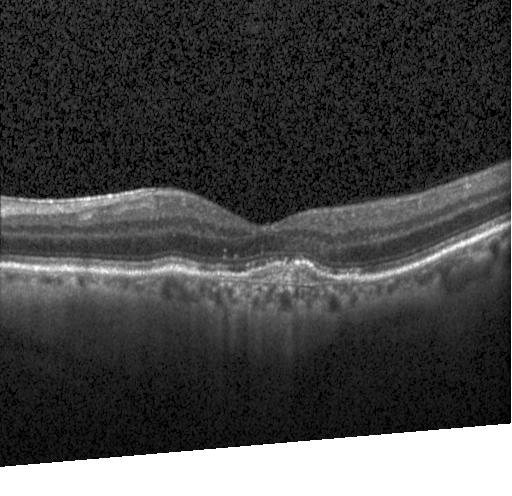 SD-OCT, OCT B-scan, horizontal scan through the fovea — This B-scan demonstrates choroidal neovascularization (CNV).